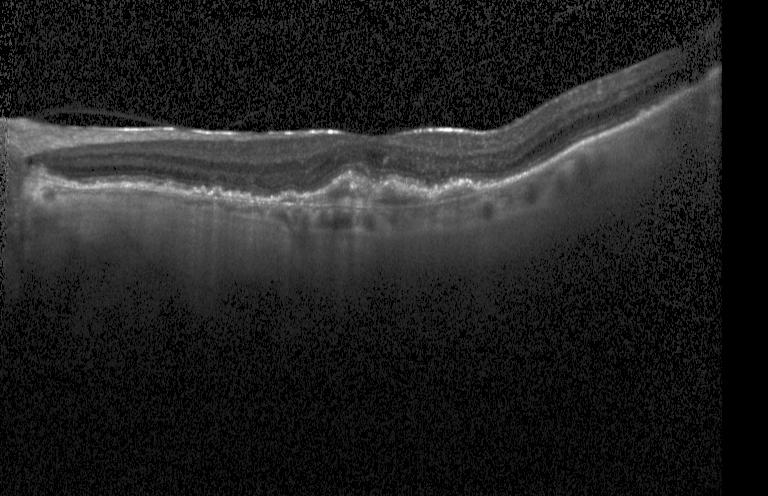

Impression: CNV.